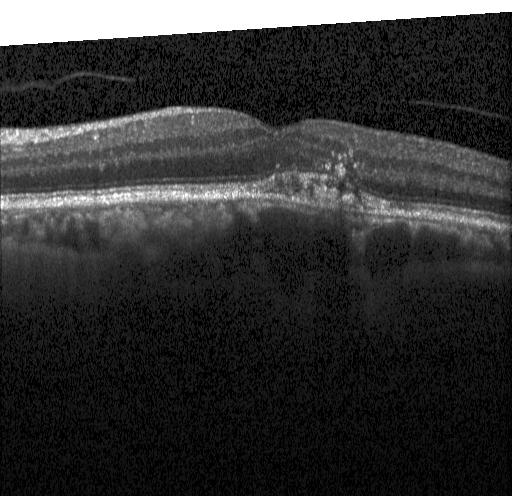
Optical coherence tomography scan — Assessment: CNV.